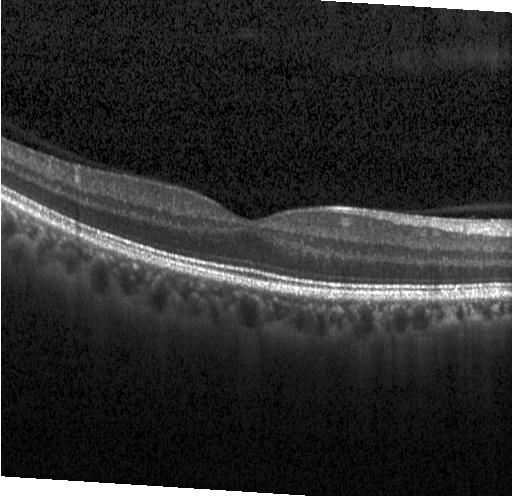

Heidelberg Spectralis, fovea-centered, SD-OCT, OCT line scan.
Finding: no choroidal neovascularization, diabetic macular edema, or drusen.